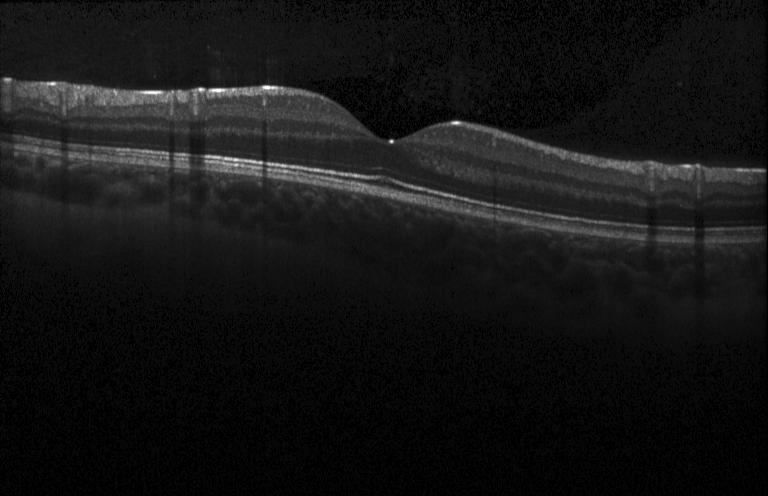
Fovea-centered. OCT B-scan. Acquired on a Heidelberg Spectralis
Impression: no evidence of choroidal neovascularization, diabetic macular edema, or drusen.